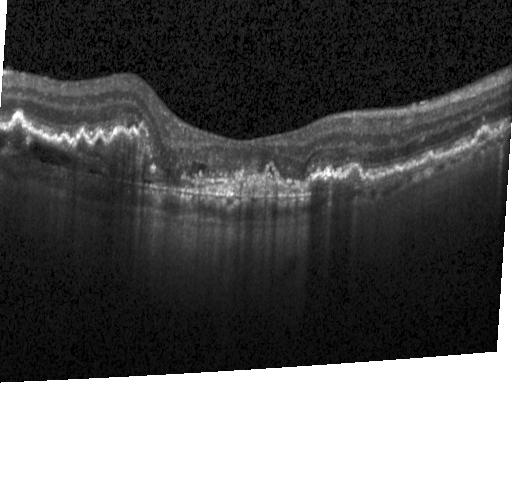
Spectral-domain OCT B-scan: choroidal neovascularization.